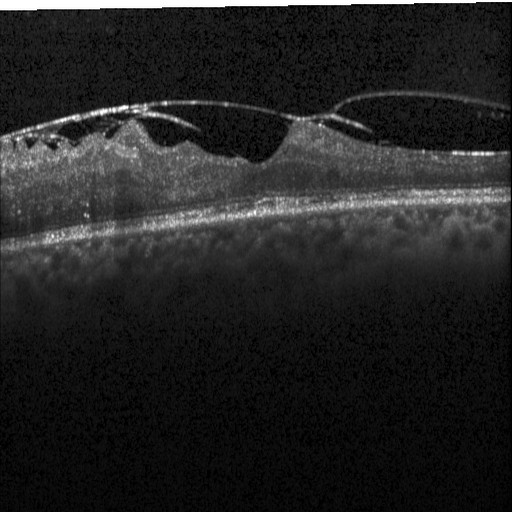
This B-scan demonstrates diabetic macular edema.